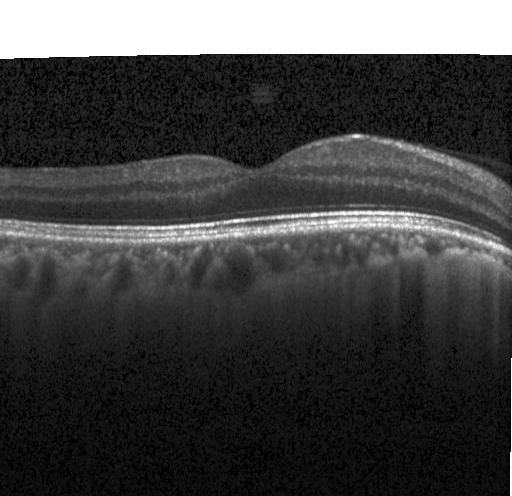

Finding: no choroidal neovascularization, diabetic macular edema, or drusen.